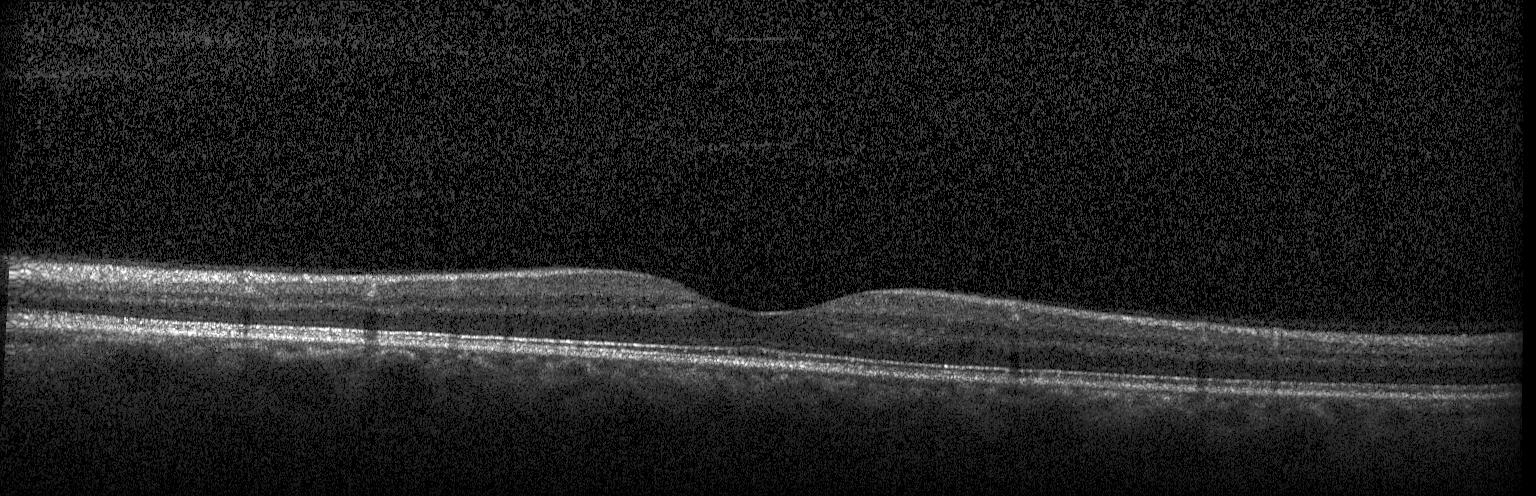

Assessment: neither choroidal neovascularization, diabetic macular edema, nor drusen.